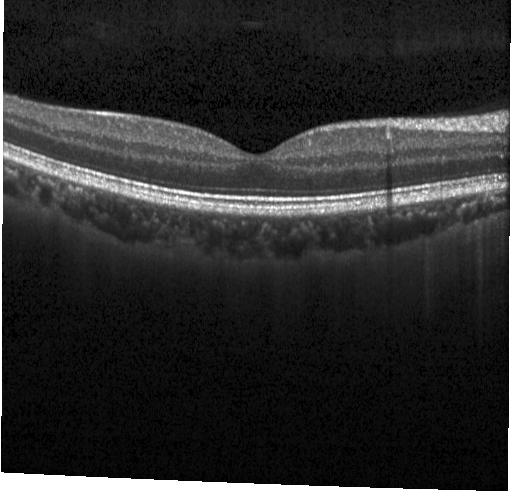 Impression: no choroidal neovascularization, diabetic macular edema, or drusen.